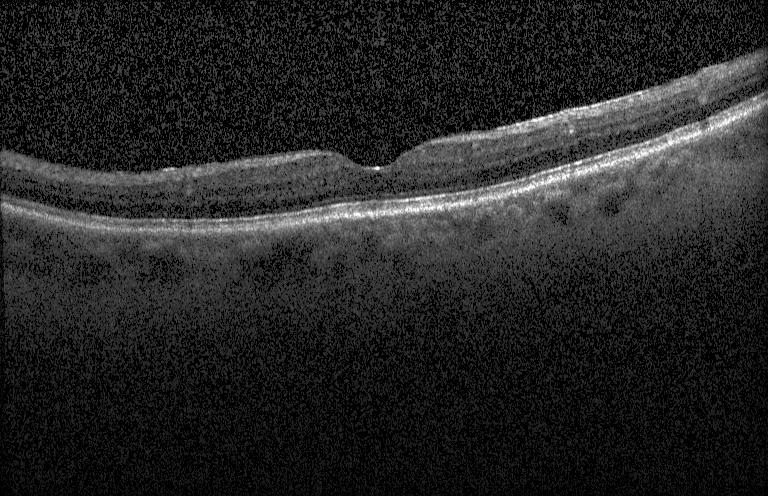
SD-OCT · horizontal scan through the fovea · optical coherence tomography scan · Heidelberg Spectralis OCT system — Diagnosis: no CNV, DME, or drusen.